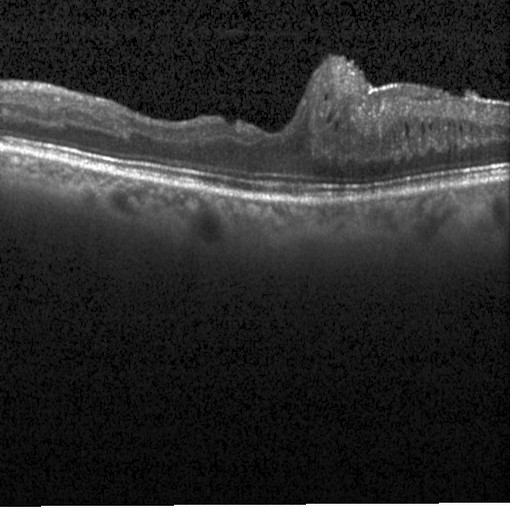
Centered on the fovea. Spectral-domain optical coherence tomography. OCT line scan. Diagnosis: DME.